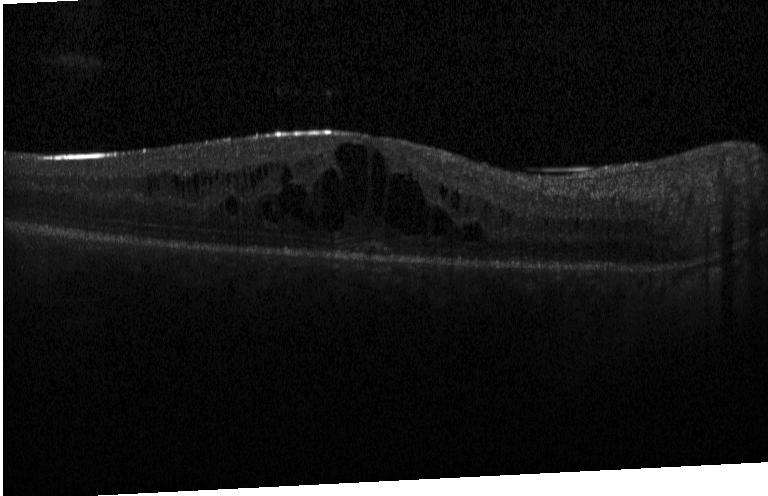 Impression: DME.